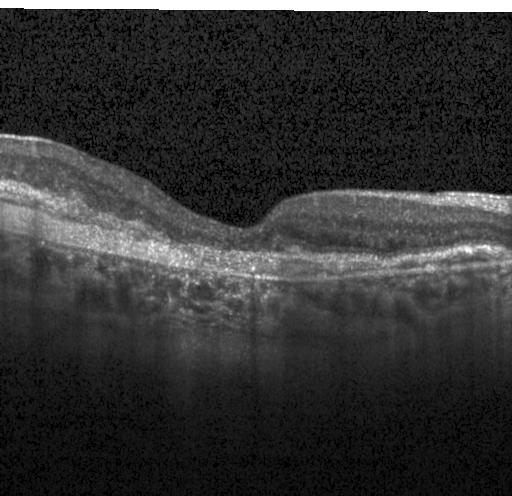
Centered on the fovea · retinal OCT B-scan — Diagnosis: a choroidal neovascular membrane.